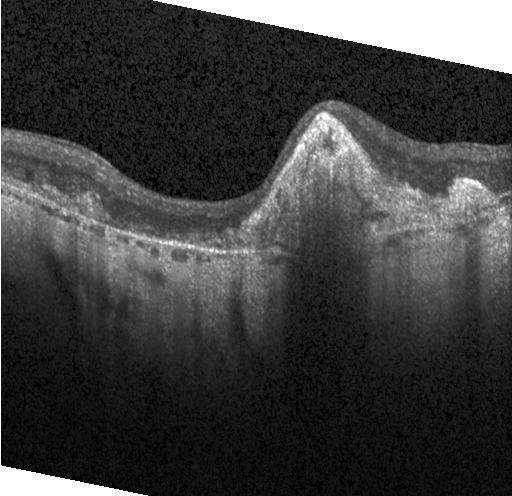 Retinal OCT B-scan — Finding: a choroidal neovascular membrane.